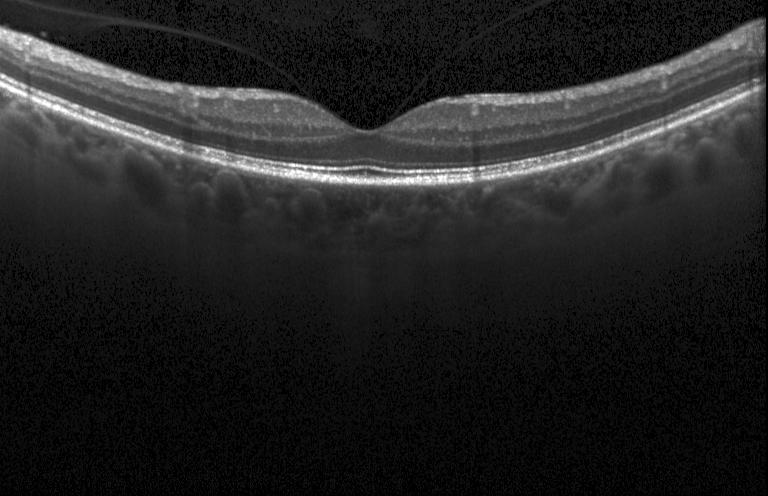 Instrument: Heidelberg Spectralis, macular scan, retinal OCT B-scan, SD-OCT — Macular OCT: no CNV, no DME, and no drusen.